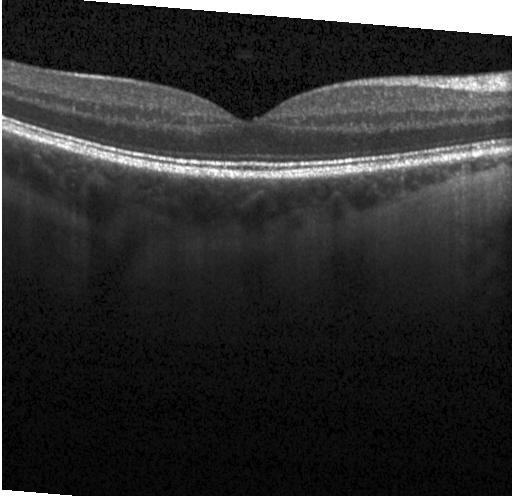

OCT B-scan showing no evidence of choroidal neovascularization, diabetic macular edema, or drusen.